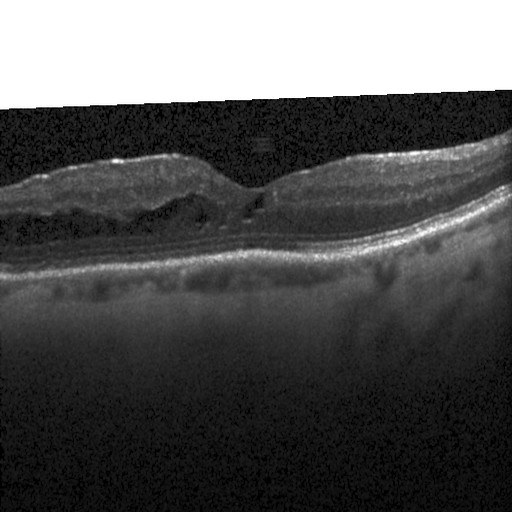

OCT scan showing diabetic macular edema (DME).